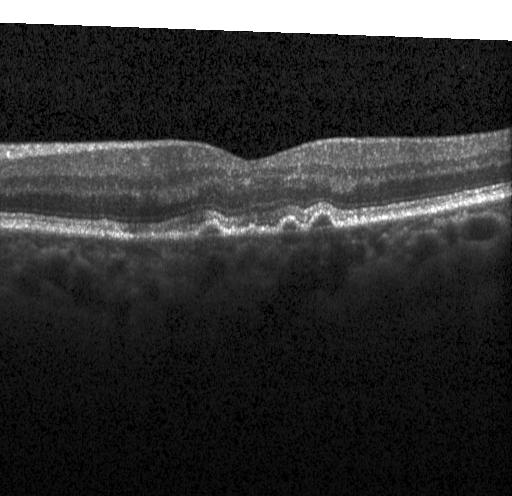

OCT finding: drusen.